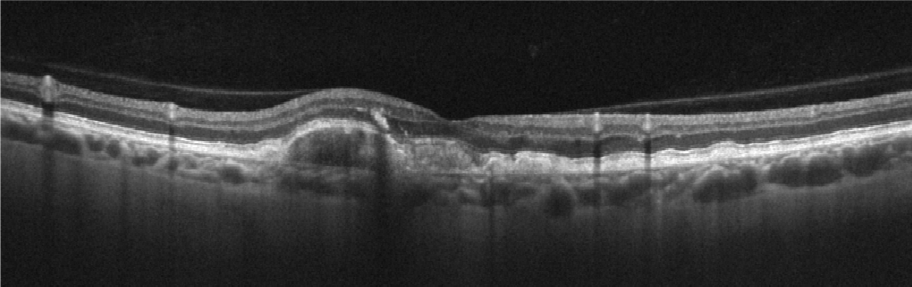 Instrument: Optovue Avanti RTVue XR. Through the macula. OCT B-scan.
Assessment: age-related macular degeneration.